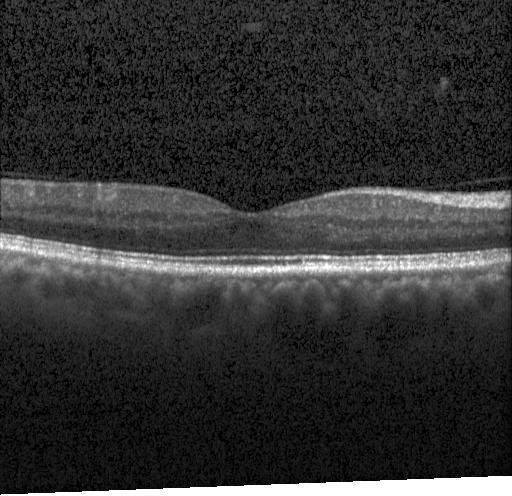

OCT line scan, Heidelberg Spectralis, spectral-domain optical coherence tomography, centered on the fovea. Finding: no evidence of CNV, DME, or drusen.